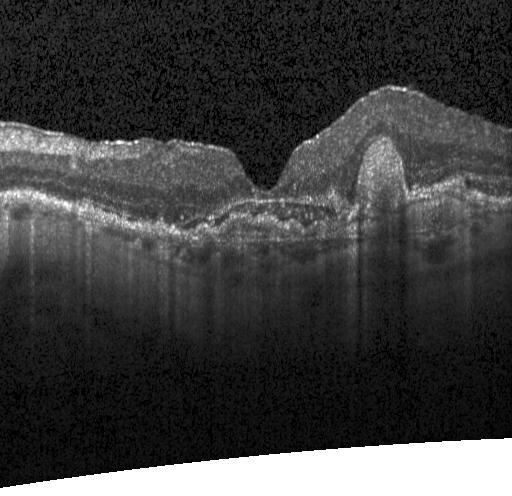

OCT line scan · through the macula — The scan shows a choroidal neovascular membrane.